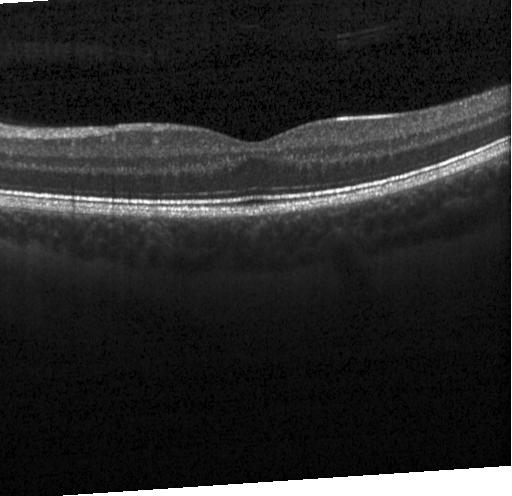
Heidelberg Spectralis; retinal OCT cross-section; macular scan; spectral-domain OCT
OCT finding: neither choroidal neovascularization, diabetic macular edema, nor drusen.